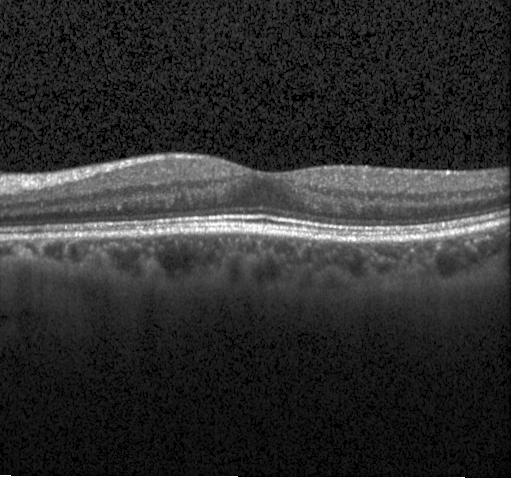
Macular OCT demonstrating neither choroidal neovascularization, diabetic macular edema, nor drusen.